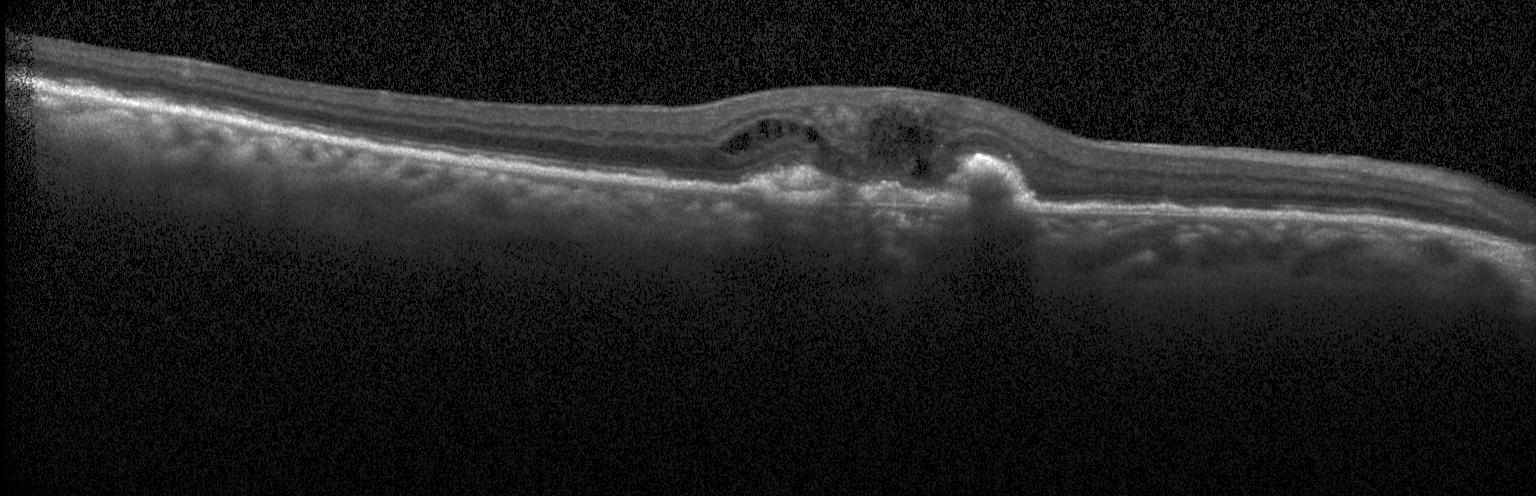 Finding: a choroidal neovascular membrane.